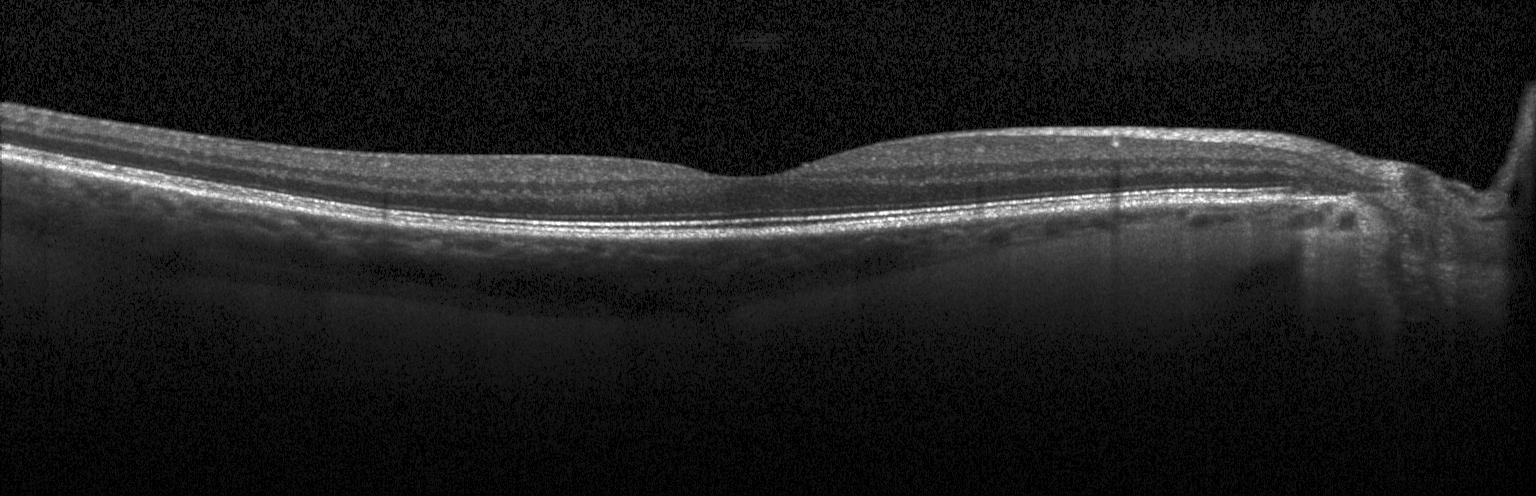
Acquired on a Heidelberg Spectralis. SD-OCT. Fovea-centered. Optical coherence tomography B-scan. Dx: no choroidal neovascularization, diabetic macular edema, or drusen.